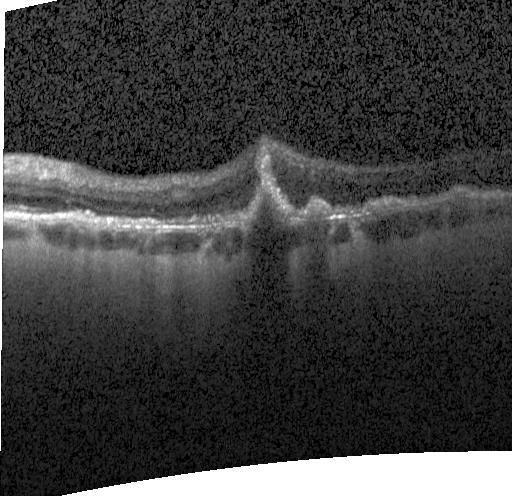 Assessment: choroidal neovascularization.